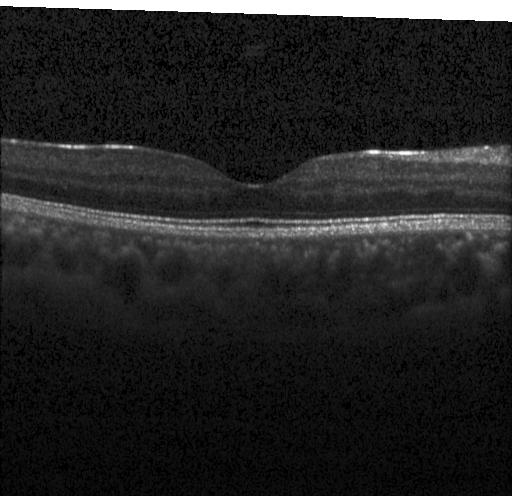 Finding: neither choroidal neovascularization, diabetic macular edema, nor drusen.